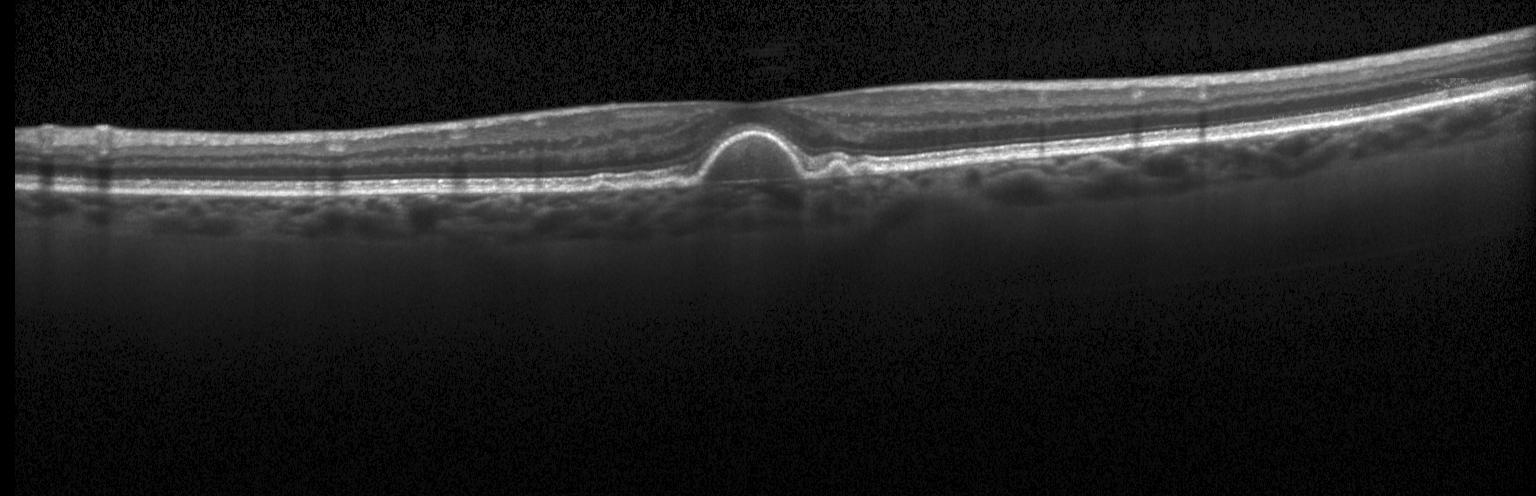

Instrument: Heidelberg Spectralis · optical coherence tomography B-scan.
The scan shows a choroidal neovascular membrane.